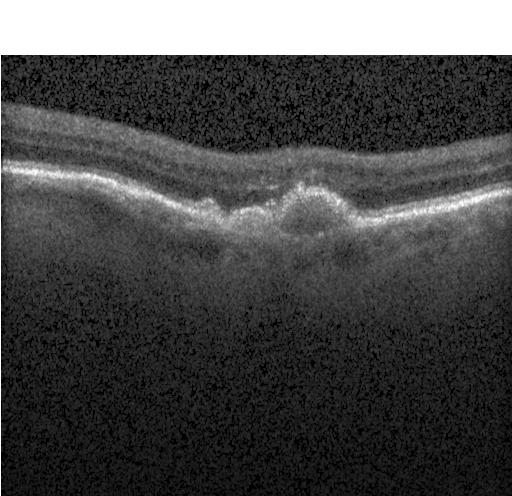 Acquired on a Heidelberg Spectralis · OCT B-scan · SD-OCT · macular scan
Assessment: a choroidal neovascular membrane.